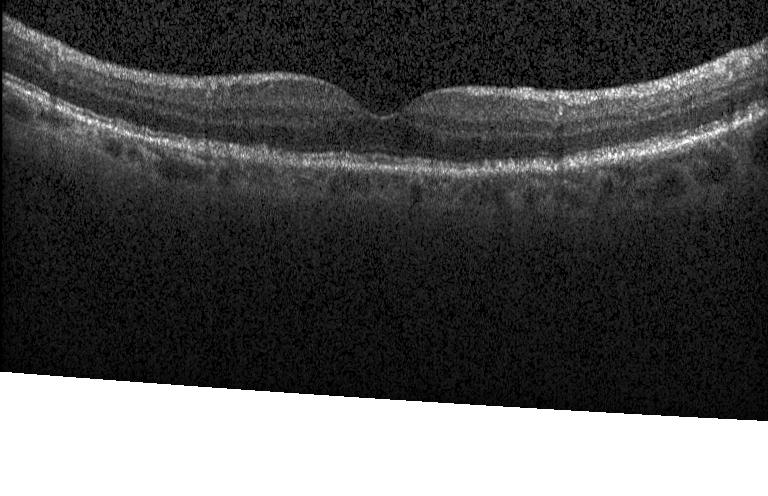
OCT line scan, spectral-domain optical coherence tomography, Heidelberg Spectralis, horizontal scan through the fovea.
Finding: drusen.